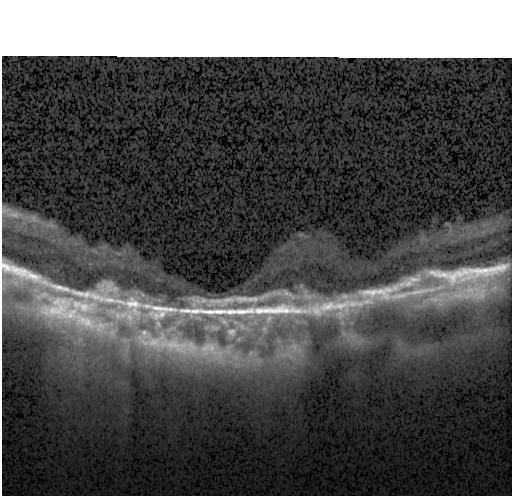
OCT line scan; instrument: Heidelberg Spectralis; spectral-domain optical coherence tomography; horizontal scan through the fovea. The scan shows a choroidal neovascular membrane.